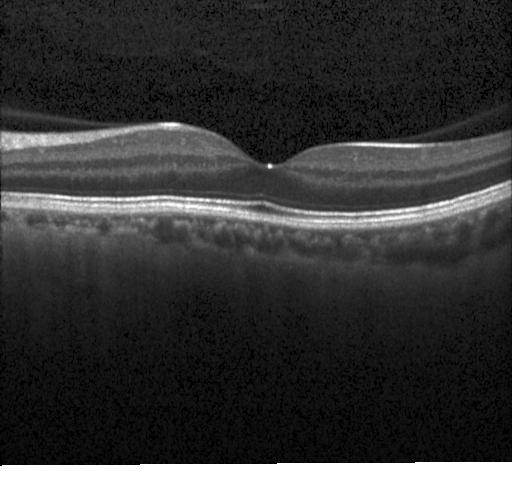

Assessment: no evidence of choroidal neovascularization, diabetic macular edema, or drusen.